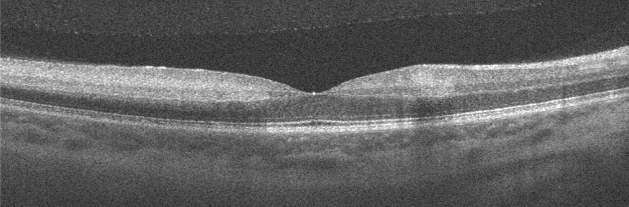
Optical coherence tomography B-scan, macular scan.
Finding: retinal artery occlusion.